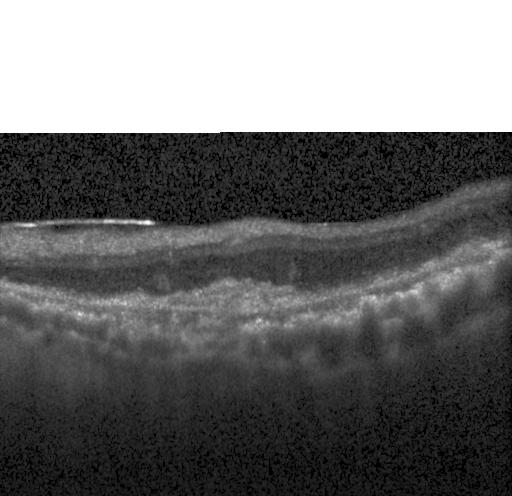
Acquired on a Heidelberg Spectralis, SD-OCT, retinal OCT cross-section, fovea-centered
OCT finding: CNV.